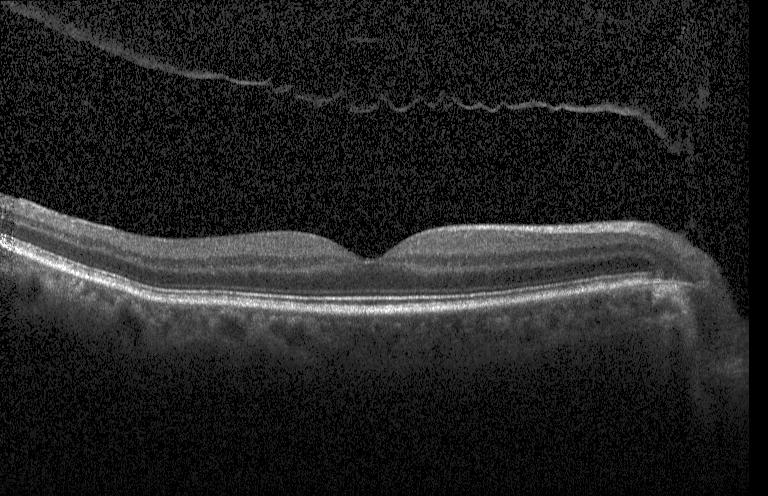

Macular OCT: no choroidal neovascularization, diabetic macular edema, or drusen.